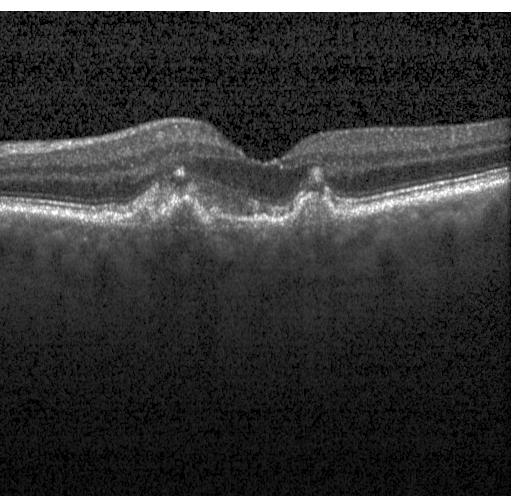

Heidelberg Spectralis. Retinal OCT B-scan. Centered on the fovea.
Macular OCT: choroidal neovascularization.